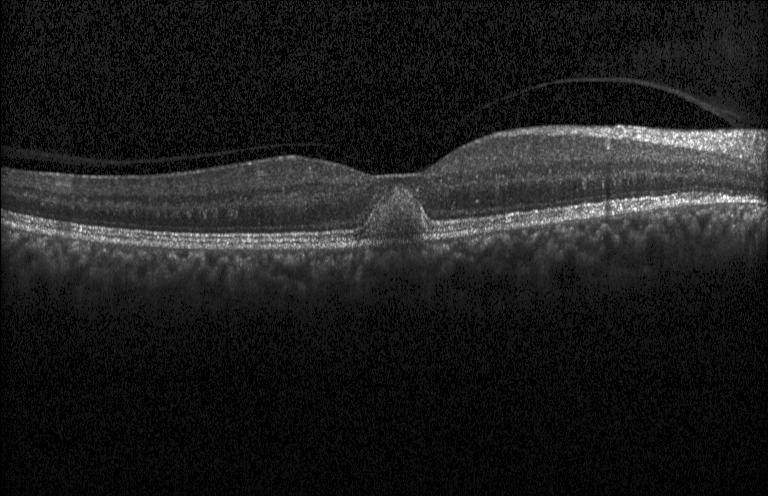
Impression: a choroidal neovascular membrane.